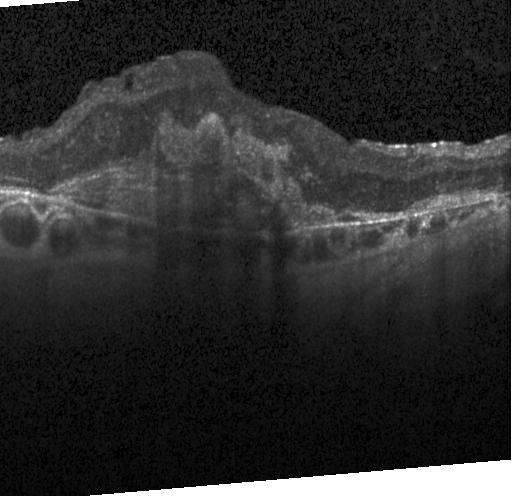

Optical coherence tomography scan, fovea-centered — Macular OCT: a choroidal neovascular membrane.